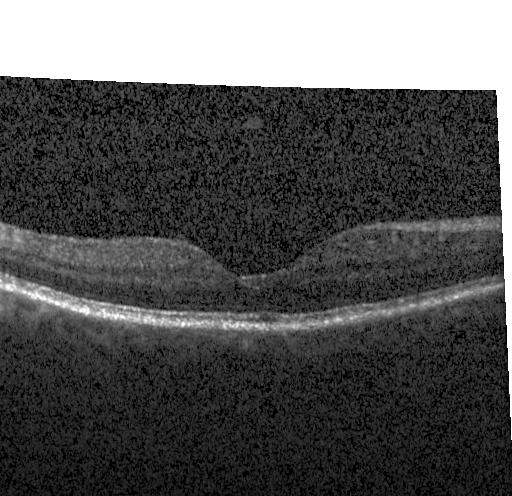

Finding: no evidence of CNV, DME, or drusen.